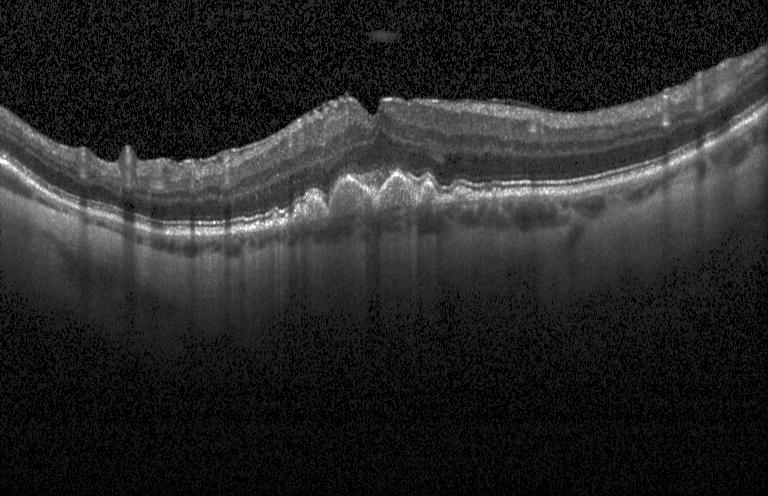

Finding: multiple drusen.